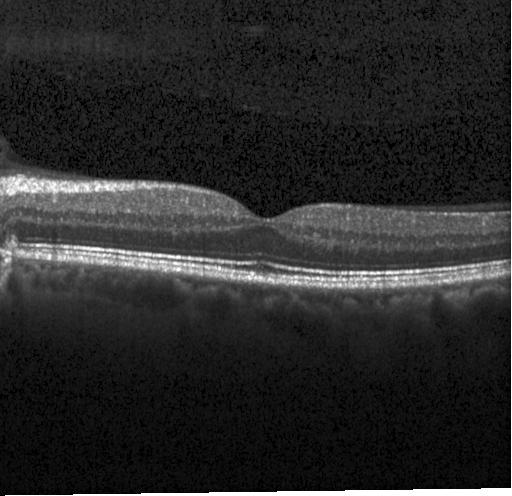
Macular OCT demonstrating no CNV, DME, or drusen.